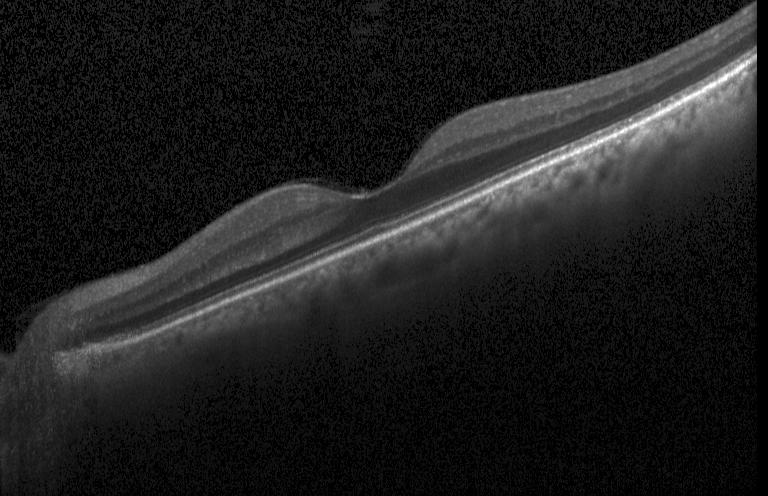 Macular scan · SD-OCT · optical coherence tomography scan · Heidelberg Spectralis OCT system — OCT finding: neither choroidal neovascularization, diabetic macular edema, nor drusen.